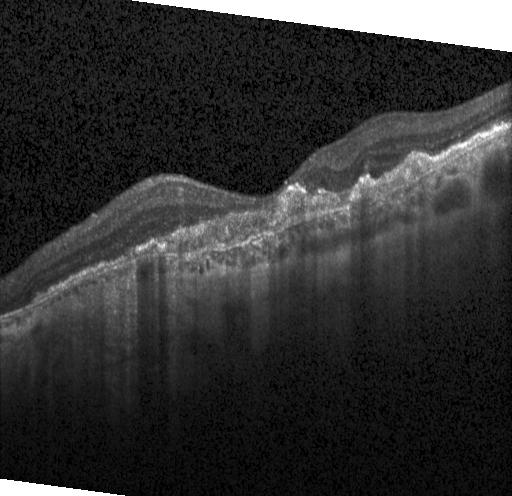

Instrument: Heidelberg Spectralis, macular scan, OCT B-scan. Impression: a choroidal neovascular membrane.